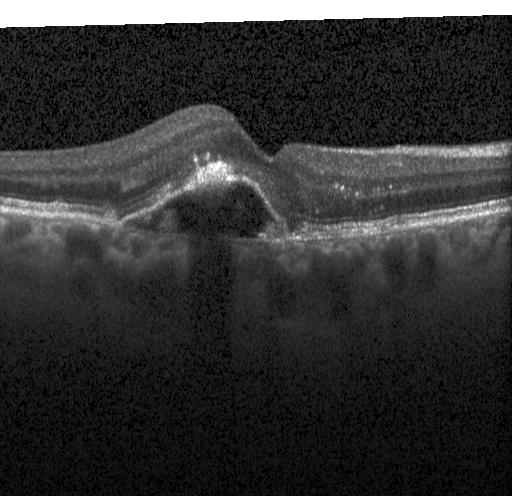 CNV.